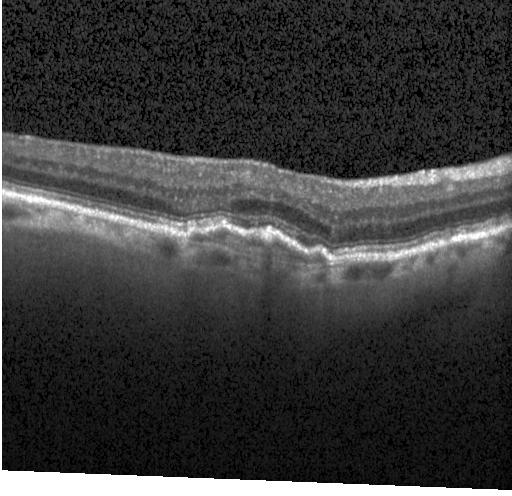
Spectral-domain OCT B-scan: choroidal neovascularization (CNV).